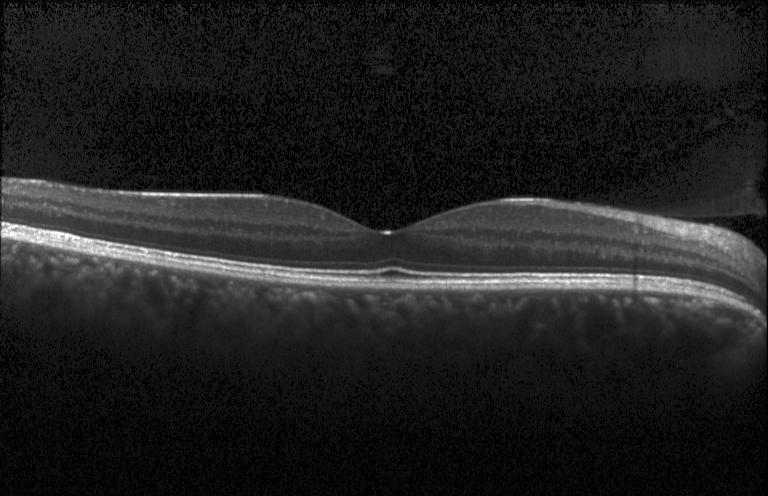 Optical coherence tomography scan — Impression: no evidence of choroidal neovascularization, diabetic macular edema, or drusen.